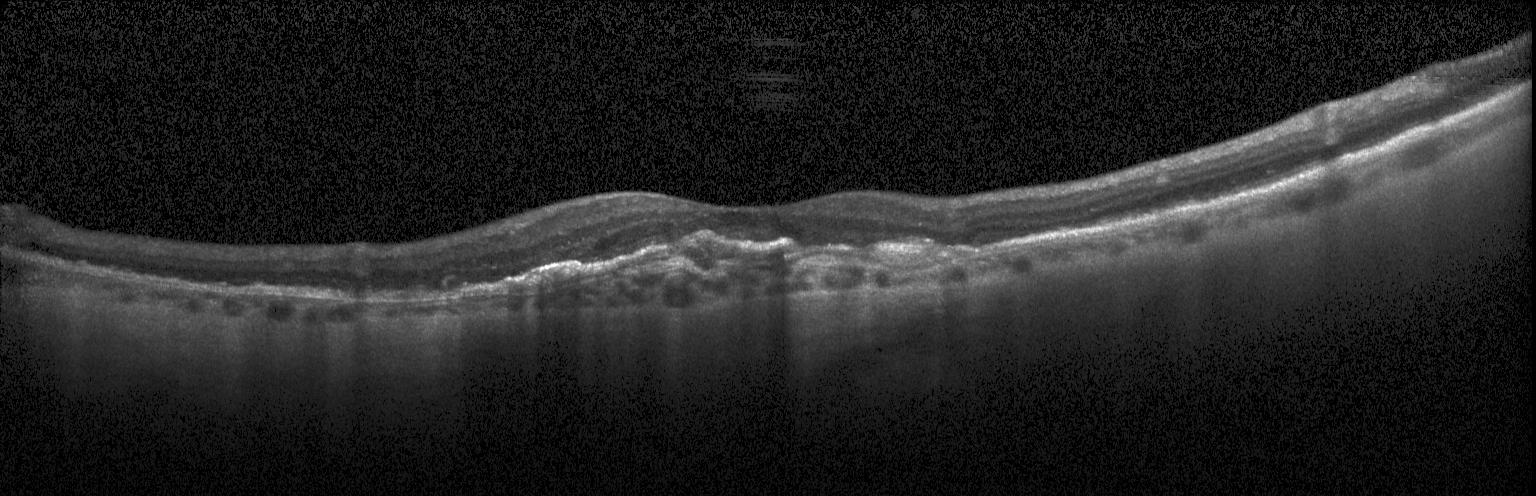
Instrument: Heidelberg Spectralis, retinal OCT B-scan, centered on the fovea — Choroidal neovascularization (CNV).